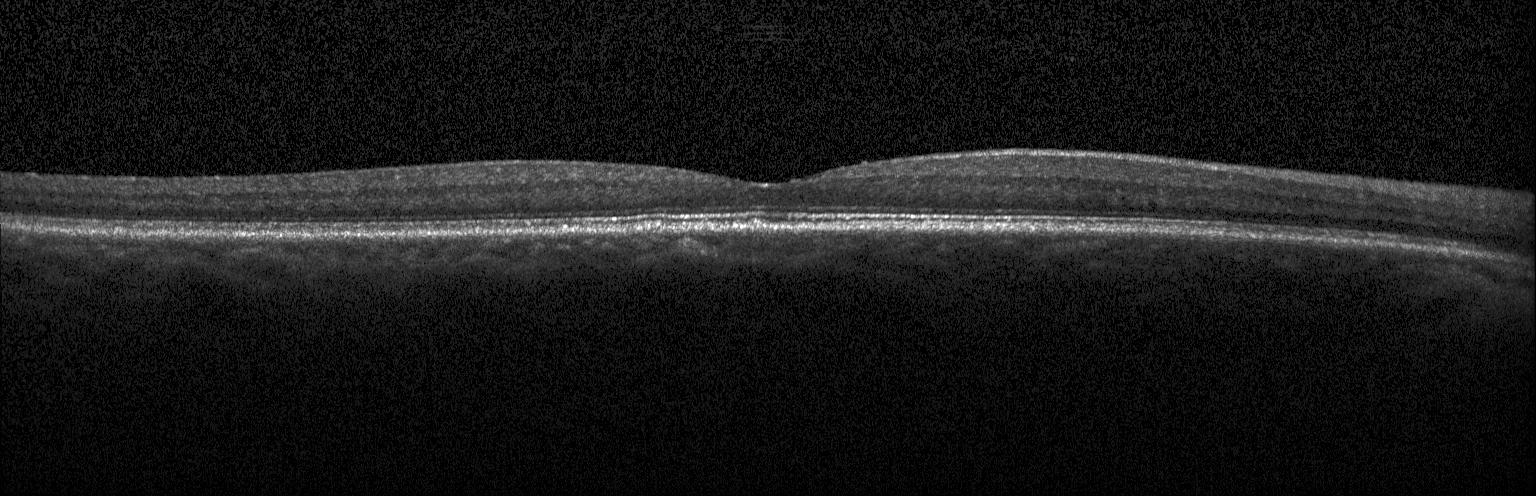

Retinal OCT B-scan. Impression: no choroidal neovascularization, diabetic macular edema, or drusen.